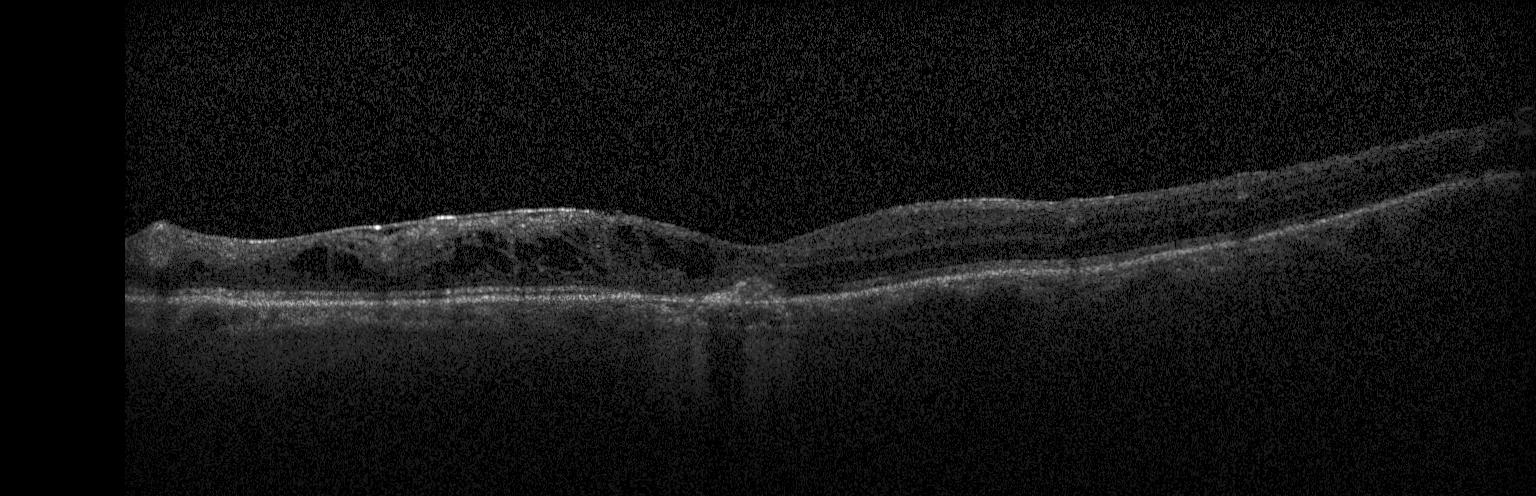

OCT B-scan — Diagnosis: a choroidal neovascular membrane.